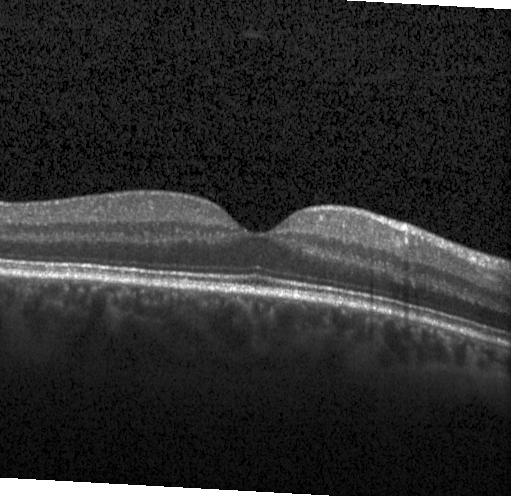

Diagnosis: no choroidal neovascularization, diabetic macular edema, or drusen.